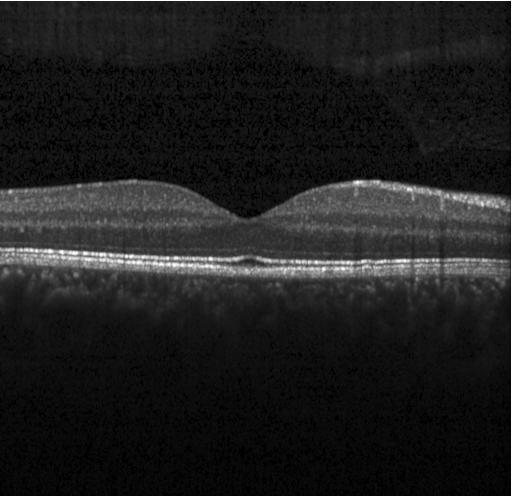

Finding: no CNV, DME, or drusen.